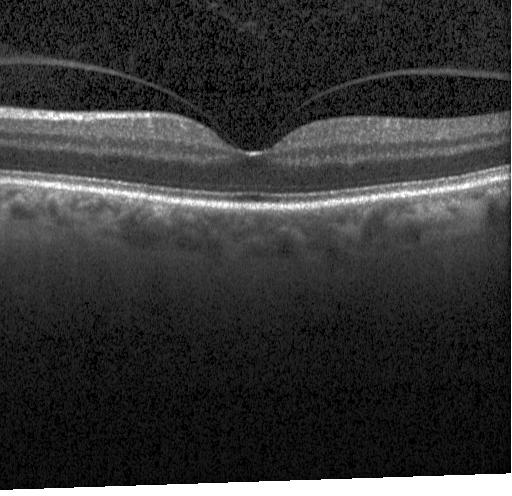 Macular OCT: no evidence of CNV, DME, or drusen.